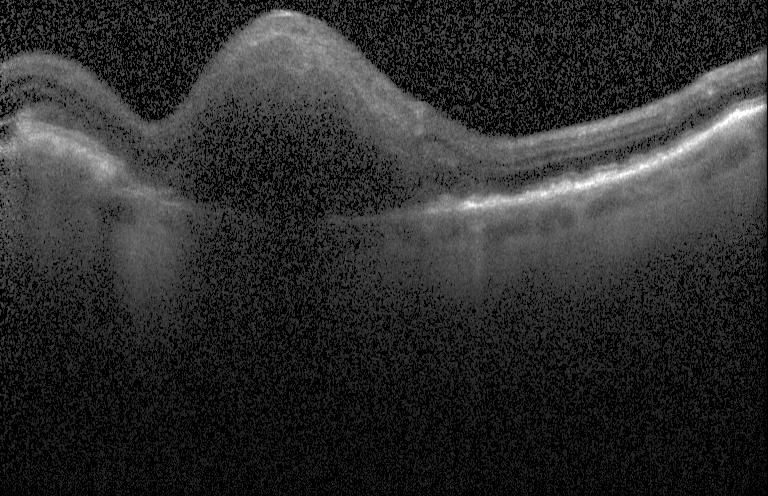

Spectral-domain OCT B-scan: a choroidal neovascular membrane.